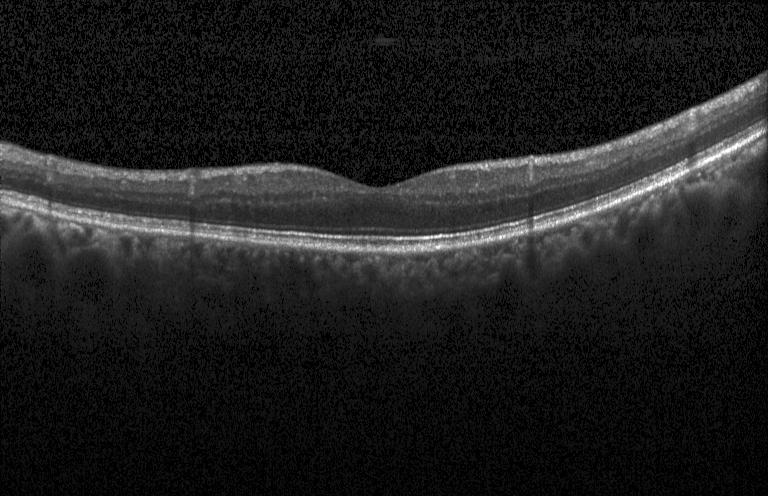 Spectral-domain OCT B-scan: no choroidal neovascularization, no diabetic macular edema, and no drusen.